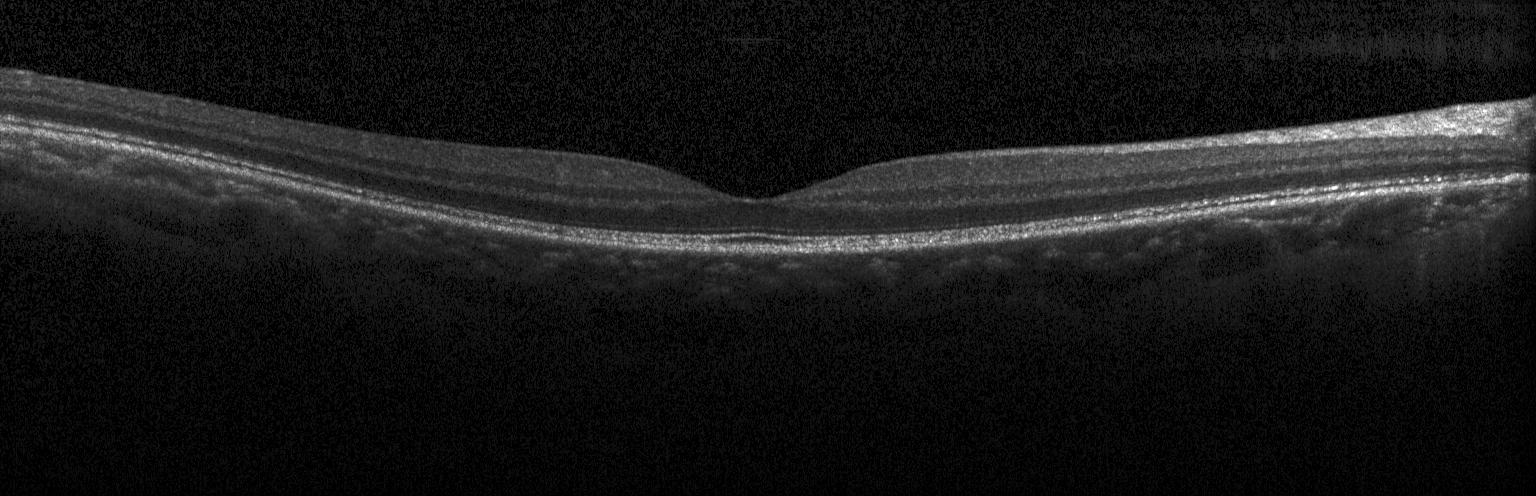

Optical coherence tomography scan. This B-scan demonstrates no evidence of choroidal neovascularization, diabetic macular edema, or drusen.